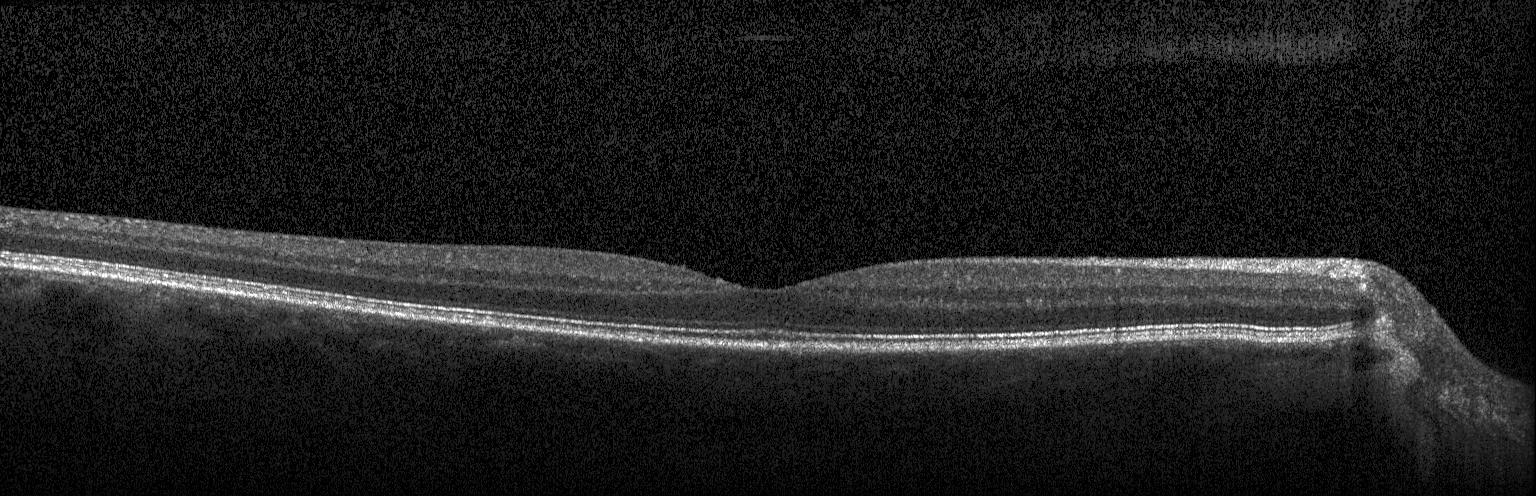 Spectral-domain optical coherence tomography · fovea-centered · OCT line scan · acquired on a Heidelberg Spectralis — Assessment: no choroidal neovascularization, no diabetic macular edema, and no drusen.